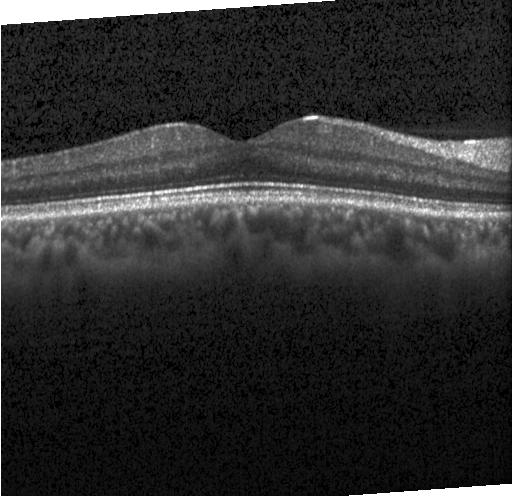

SD-OCT · optical coherence tomography B-scan · Heidelberg Spectralis. This B-scan demonstrates no choroidal neovascularization, no diabetic macular edema, and no drusen.